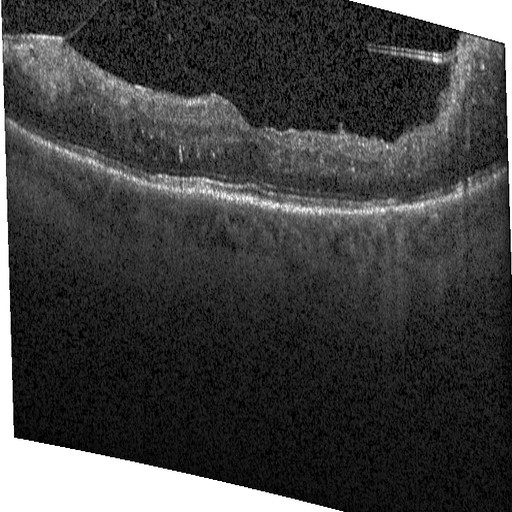 OCT finding: DME.